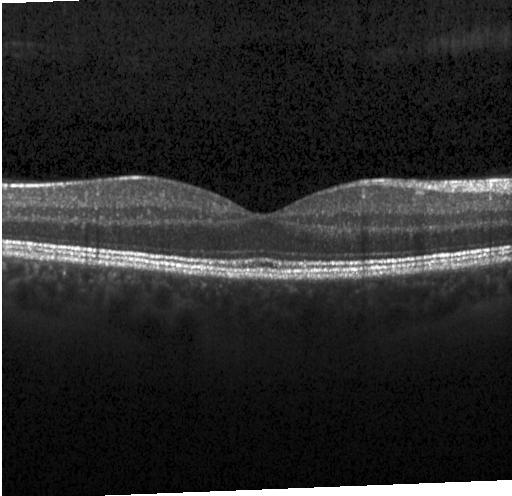

OCT B-scan. Fovea-centered — Dx: no evidence of choroidal neovascularization, diabetic macular edema, or drusen.